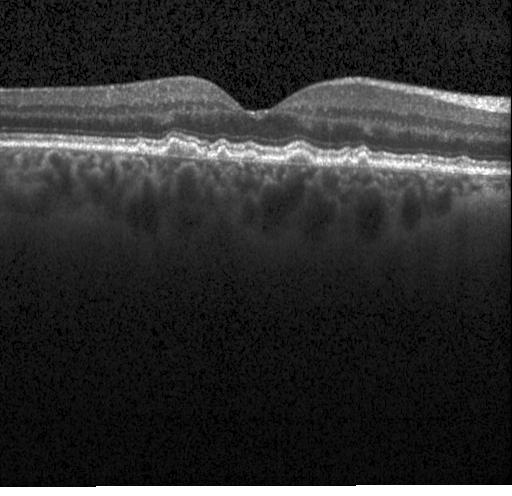

Through the macula, retinal OCT B-scan
Finding: sub-RPE drusenoid deposits.